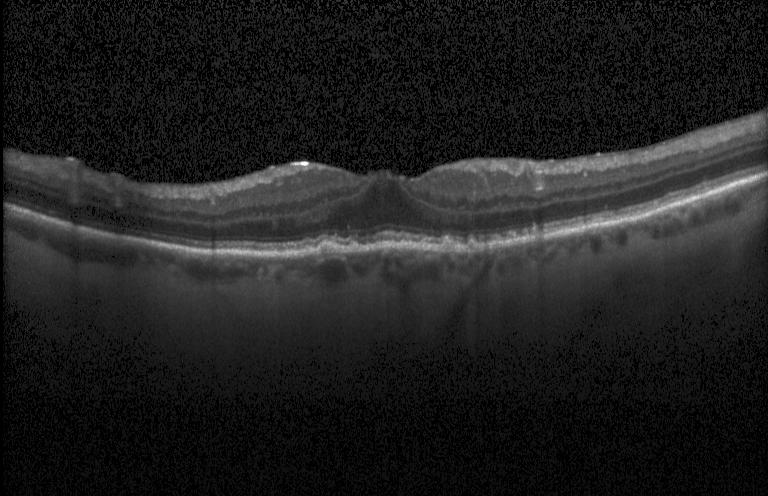

Retinal OCT B-scan; spectral-domain optical coherence tomography; instrument: Heidelberg Spectralis — Impression: sub-RPE drusenoid deposits.